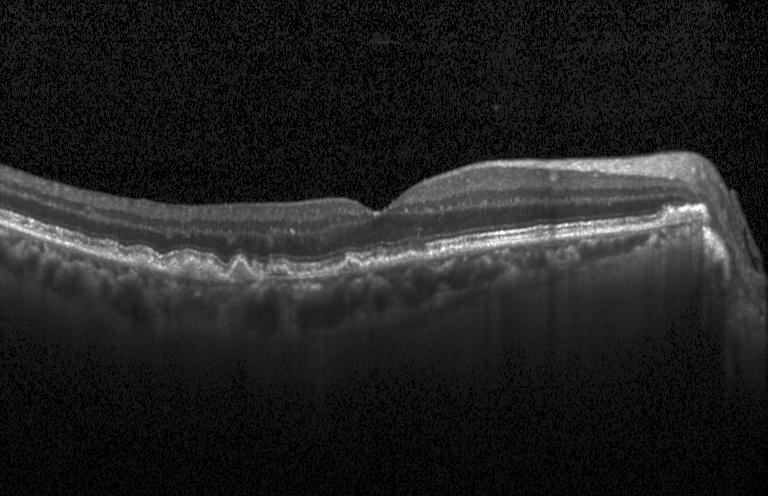

Macular scan. Heidelberg Spectralis OCT system. Retinal OCT B-scan. Spectral-domain OCT. This B-scan demonstrates drusen.